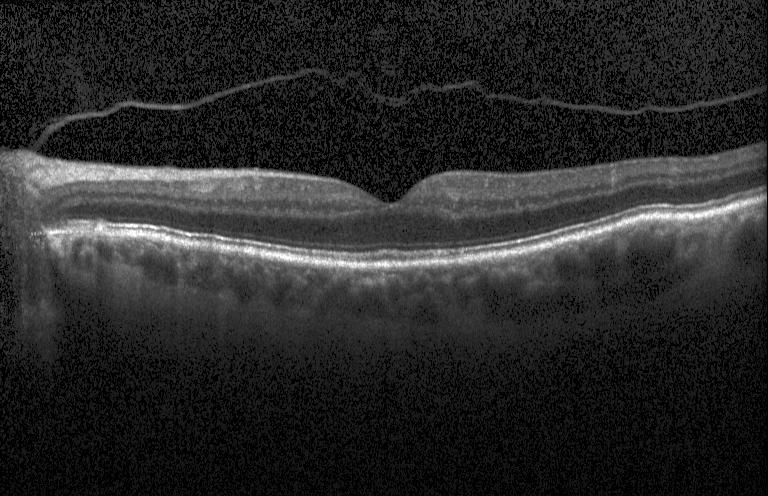
Fovea-centered; Heidelberg Spectralis OCT system; OCT line scan; spectral-domain optical coherence tomography
The scan shows no choroidal neovascularization, diabetic macular edema, or drusen.